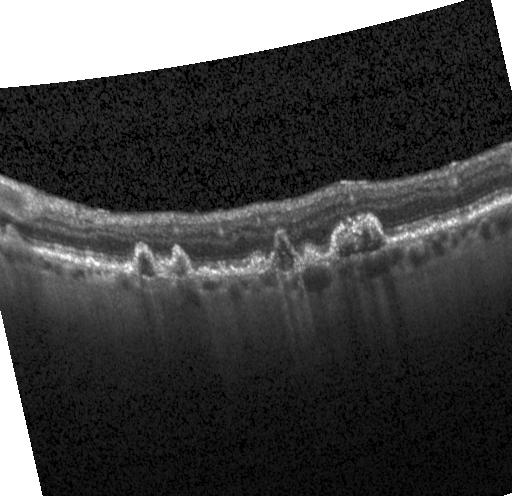 Optical coherence tomography scan · instrument: Heidelberg Spectralis · fovea-centered · spectral-domain OCT
Macular OCT: CNV.